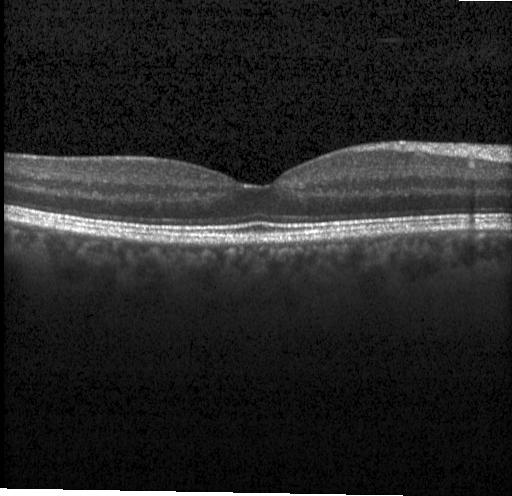

Acquired on a Heidelberg Spectralis. Macular scan. OCT B-scan.
Finding: neither CNV, DME, nor drusen.